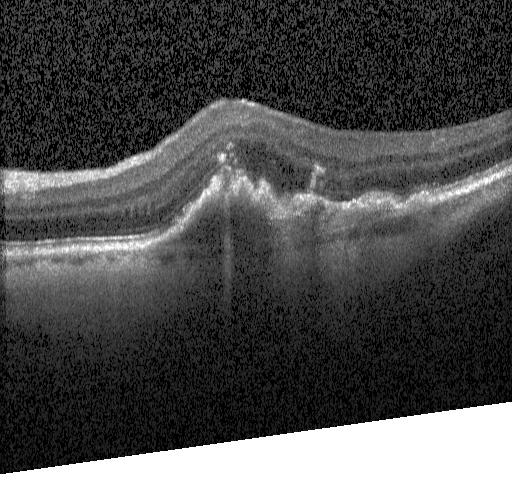
Impression: a choroidal neovascular membrane.